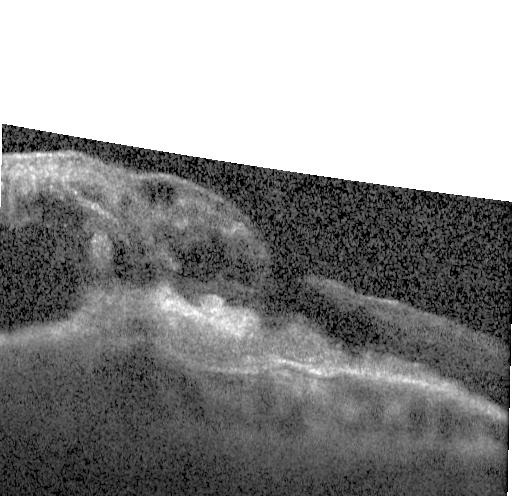
Heidelberg Spectralis, retinal OCT cross-section
A choroidal neovascular membrane.